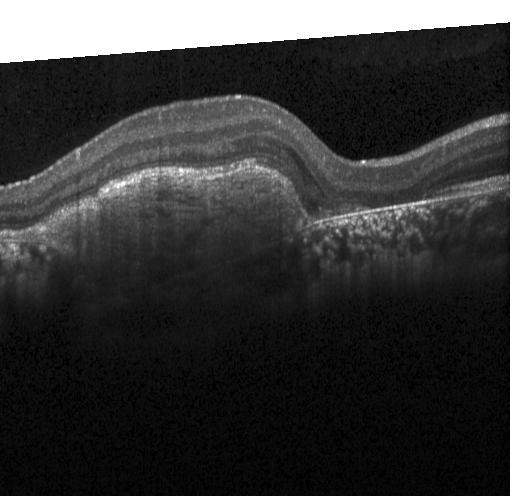
Acquired on a Heidelberg Spectralis; fovea-centered; spectral-domain OCT; OCT line scan
Impression: a choroidal neovascular membrane.